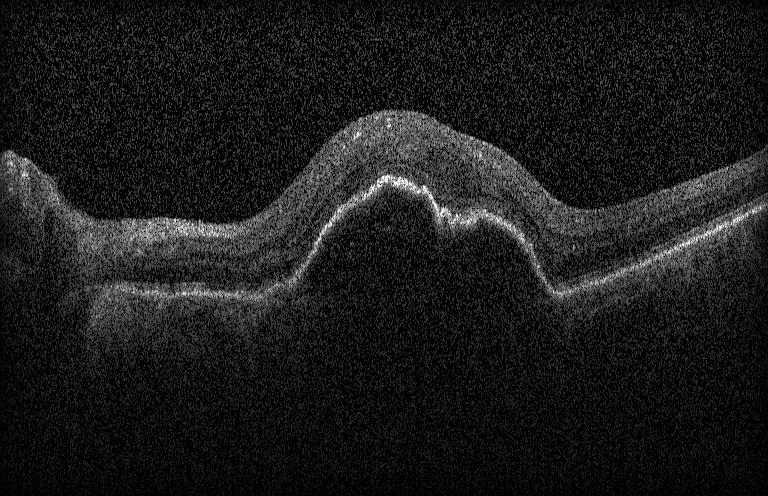
The scan shows choroidal neovascularization.